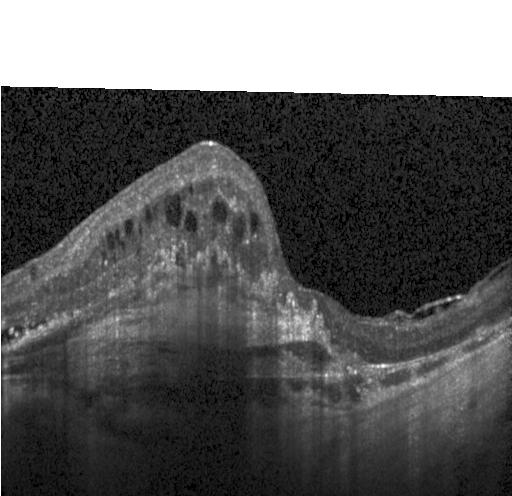 Spectral-domain OCT · retinal OCT cross-section · acquired on a Heidelberg Spectralis — This B-scan demonstrates CNV.